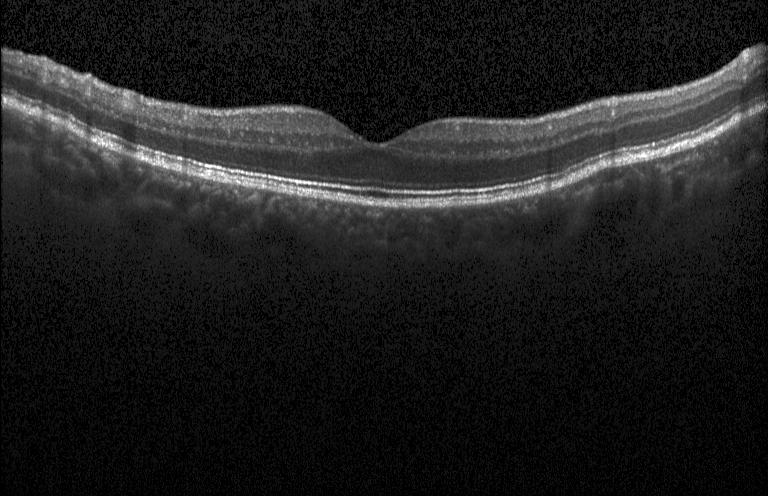 SD-OCT; optical coherence tomography B-scan
Impression: no choroidal neovascularization, diabetic macular edema, or drusen.